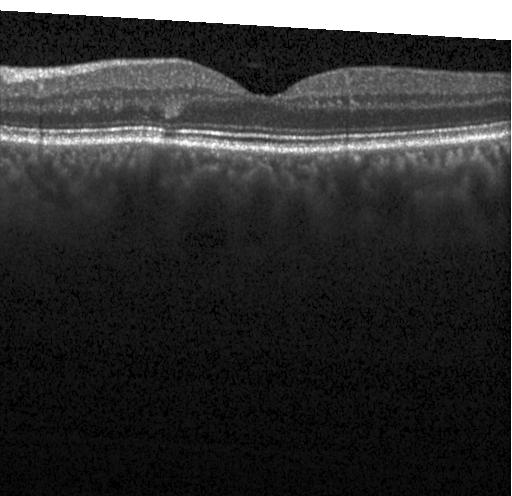 Acquired on a Heidelberg Spectralis. SD-OCT. Macular scan. Optical coherence tomography B-scan. Macular OCT: no choroidal neovascularization, no diabetic macular edema, and no drusen.